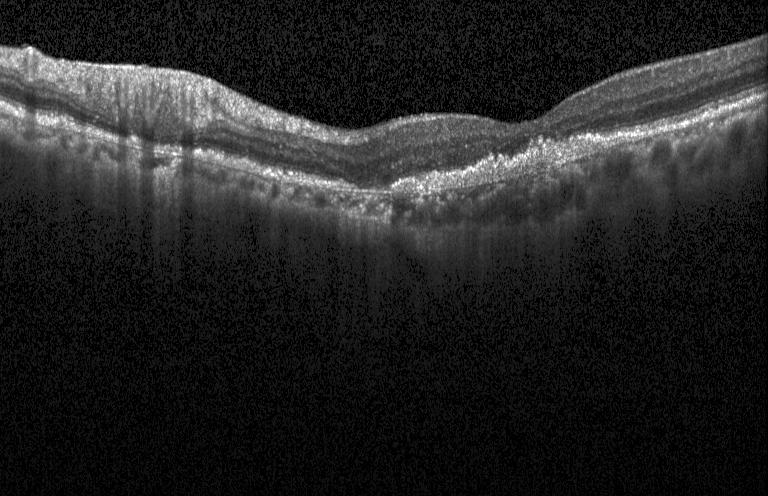 Spectral-domain OCT B-scan: CNV.